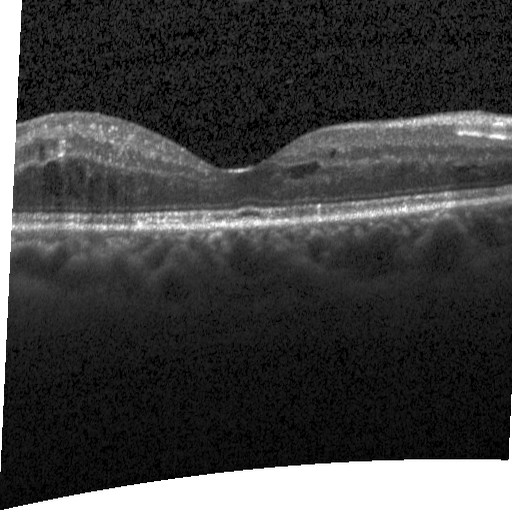

Assessment: DME.